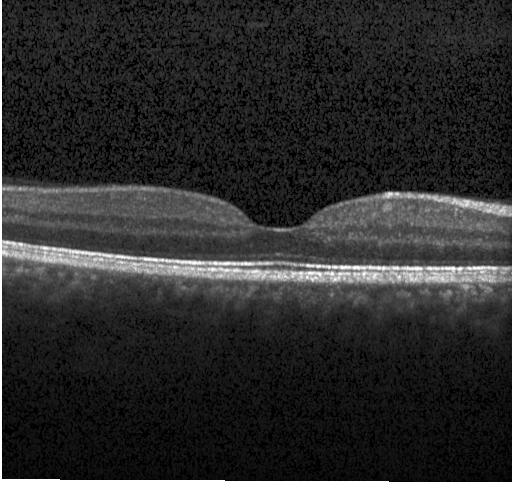
SD-OCT; centered on the fovea; OCT line scan.
Impression: neither choroidal neovascularization, diabetic macular edema, nor drusen.